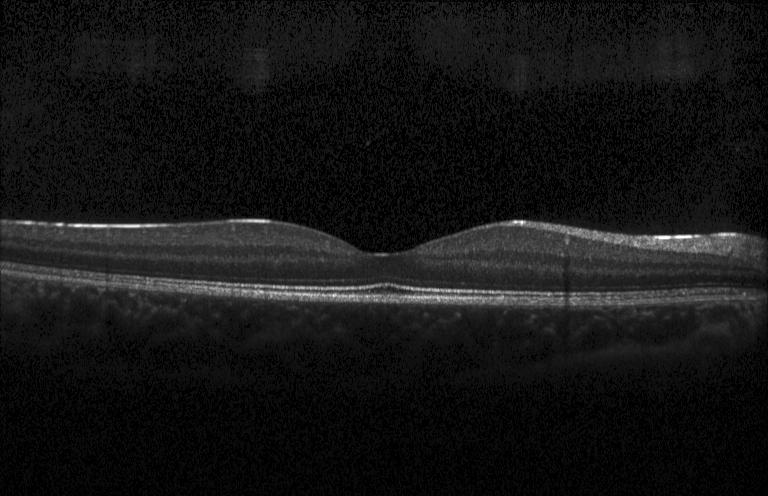
Spectral-domain OCT; OCT B-scan — Impression: no evidence of choroidal neovascularization, diabetic macular edema, or drusen.